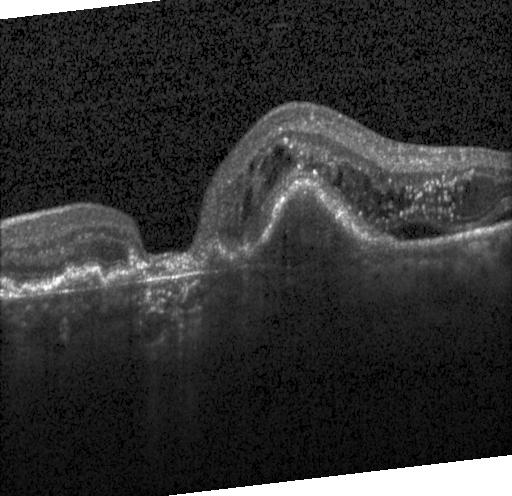

Instrument: Heidelberg Spectralis. Centered on the fovea. SD-OCT. OCT B-scan
This B-scan demonstrates CNV.